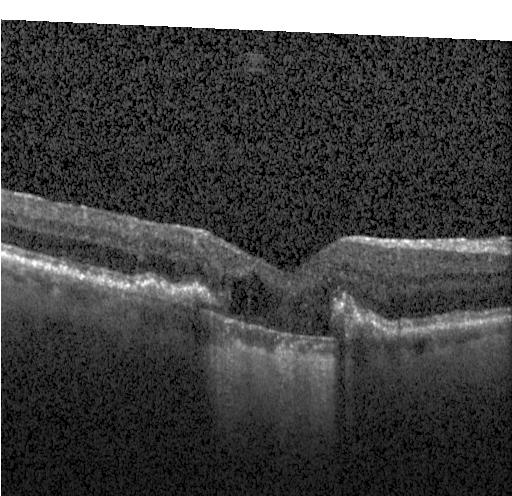

Impression: a choroidal neovascular membrane.